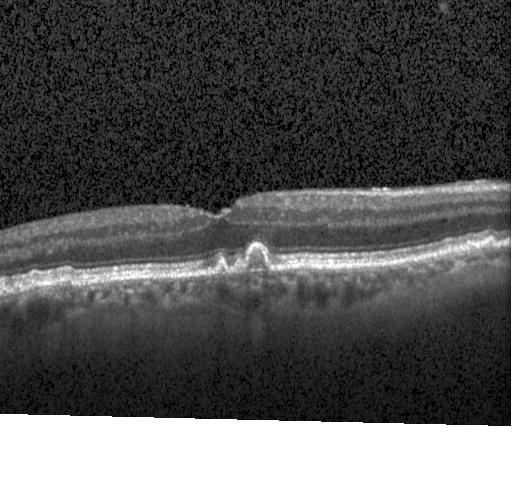
The scan shows multiple drusen.